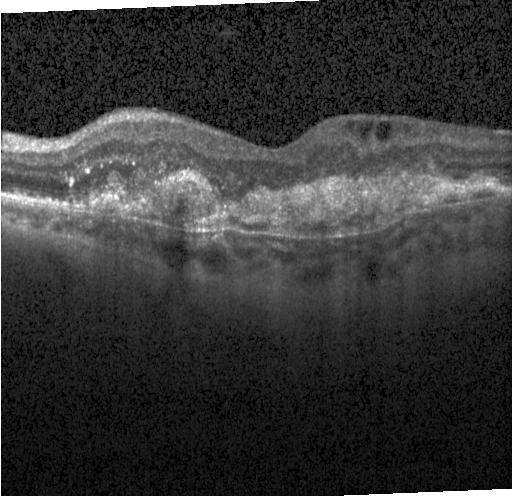

Retinal OCT B-scan. Instrument: Heidelberg Spectralis. Spectral-domain OCT. Fovea-centered. Finding: choroidal neovascularization (CNV).